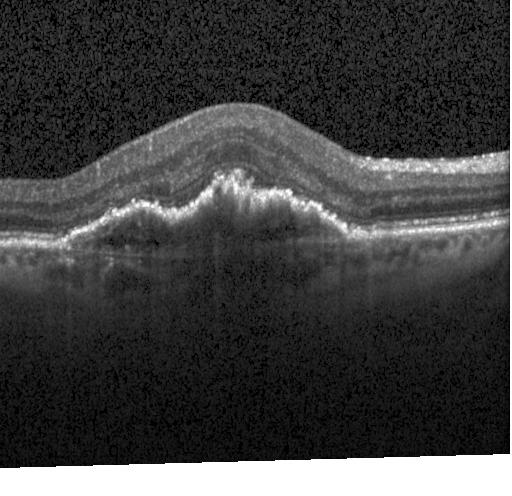

Impression: a choroidal neovascular membrane.